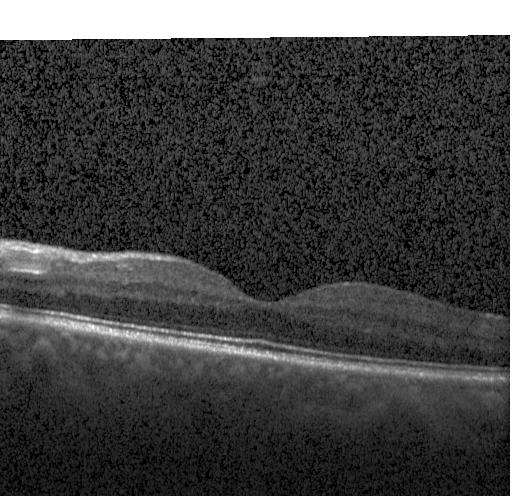
SD-OCT · retinal OCT cross-section.
Impression: neither choroidal neovascularization, diabetic macular edema, nor drusen.